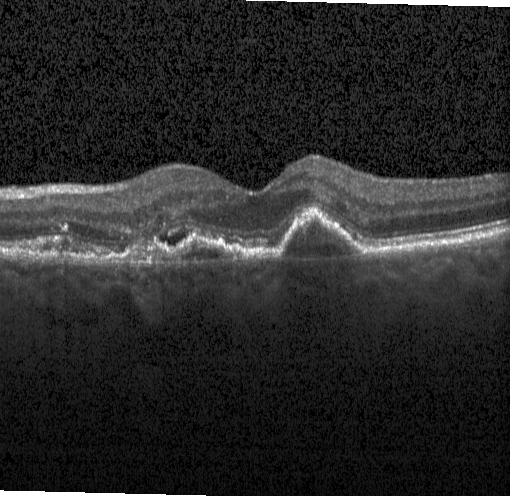 Heidelberg Spectralis, spectral-domain optical coherence tomography, fovea-centered, OCT line scan.
Macular OCT: choroidal neovascularization (CNV).